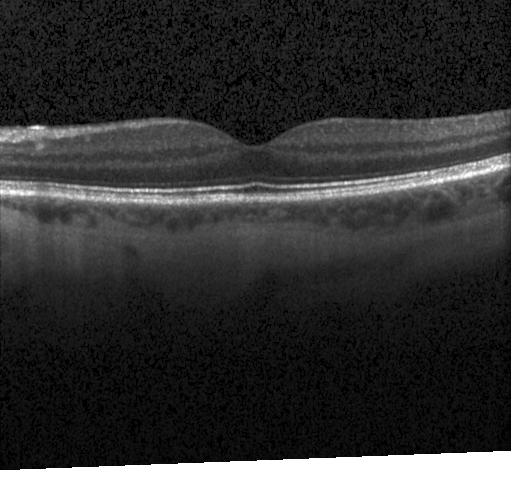 Optical coherence tomography B-scan
The scan shows no choroidal neovascularization, no diabetic macular edema, and no drusen.